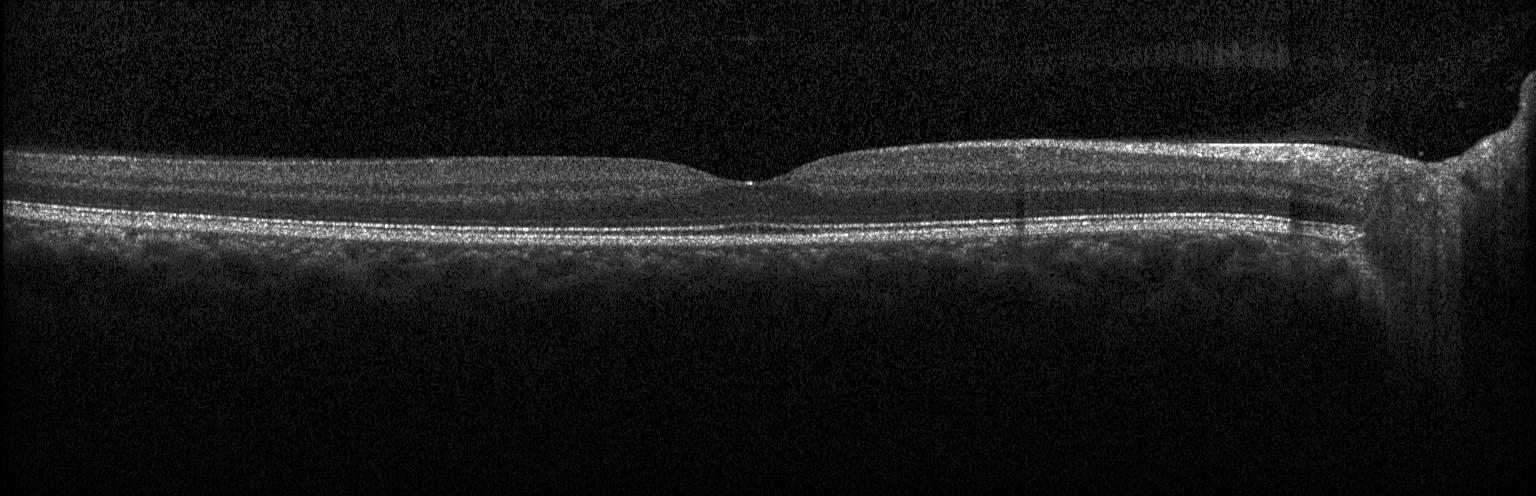 Retinal OCT cross-section; Heidelberg Spectralis.
Finding: neither choroidal neovascularization, diabetic macular edema, nor drusen.